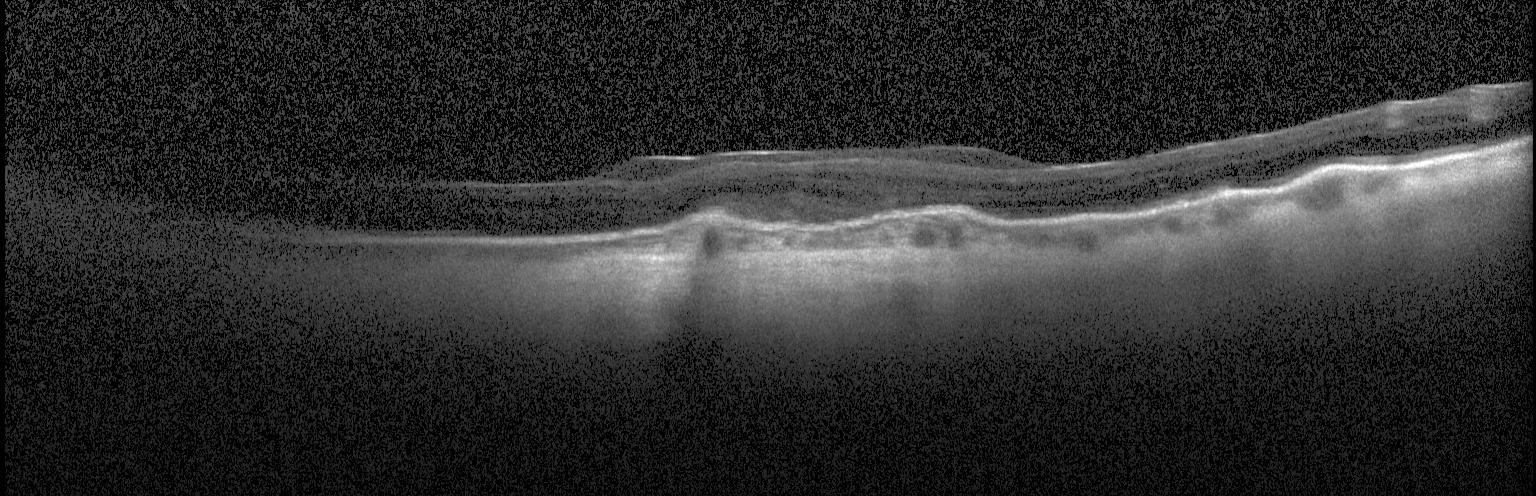
Impression: a choroidal neovascular membrane.